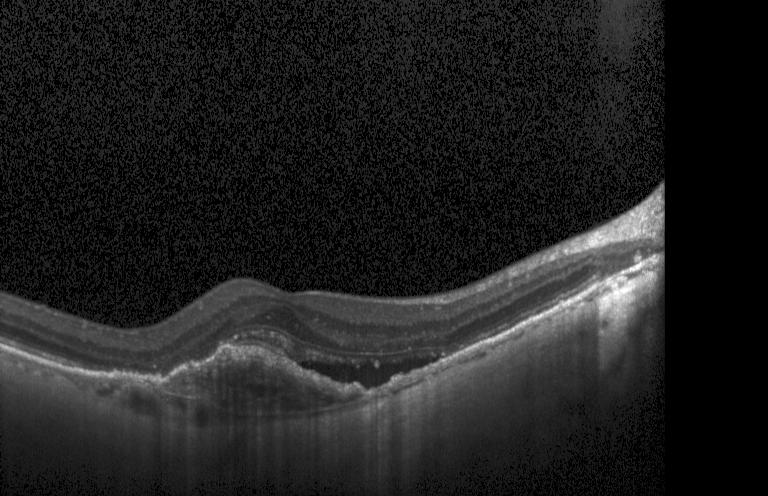
OCT B-scan showing a choroidal neovascular membrane.